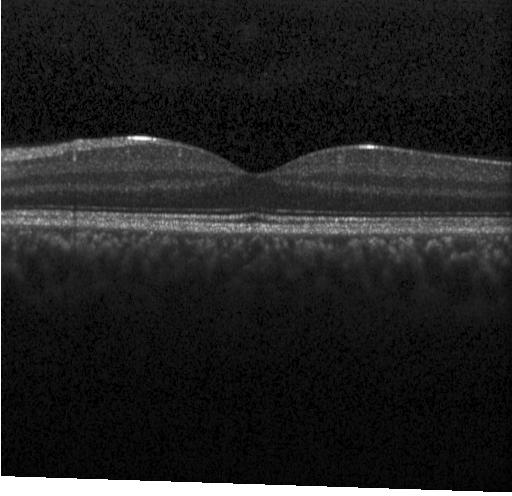 Optical coherence tomography scan · macular scan.
Dx: no choroidal neovascularization, no diabetic macular edema, and no drusen.